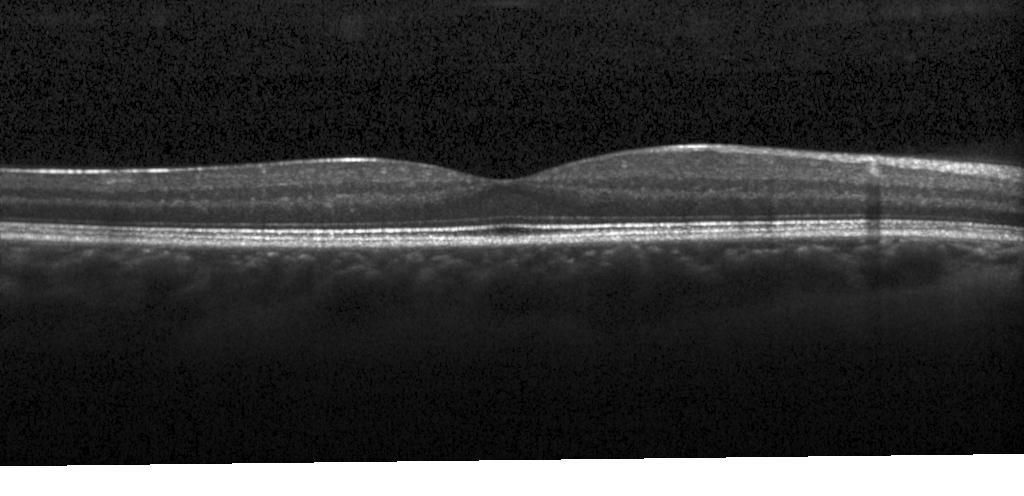
Centered on the fovea, retinal OCT cross-section
Diagnosis: no evidence of choroidal neovascularization, diabetic macular edema, or drusen.